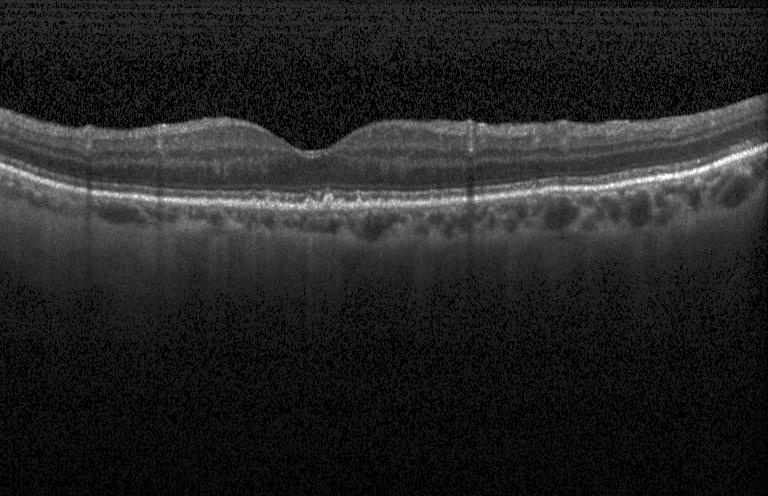 Impression: drusen.